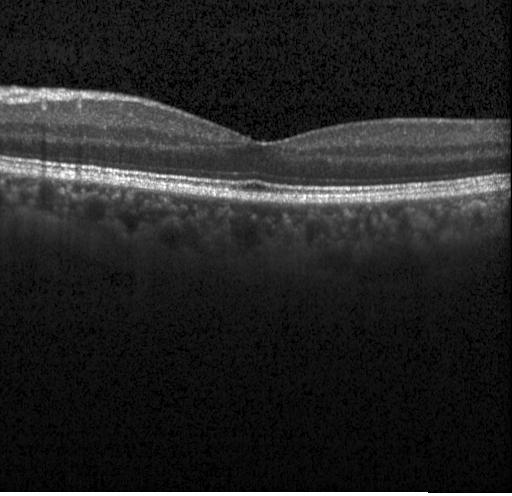
Optical coherence tomography scan. Spectral-domain optical coherence tomography. Diagnosis: no choroidal neovascularization, diabetic macular edema, or drusen.